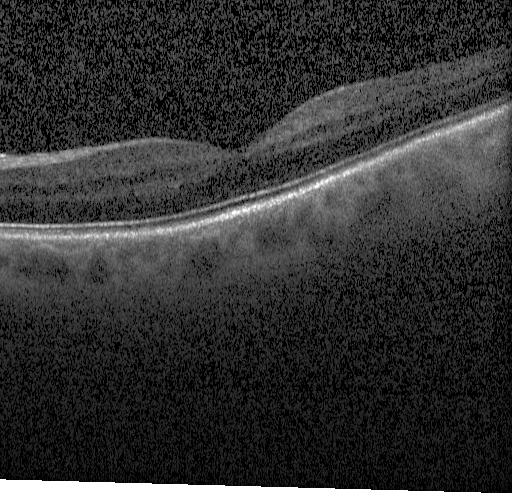

The scan shows no CNV, no DME, and no drusen.